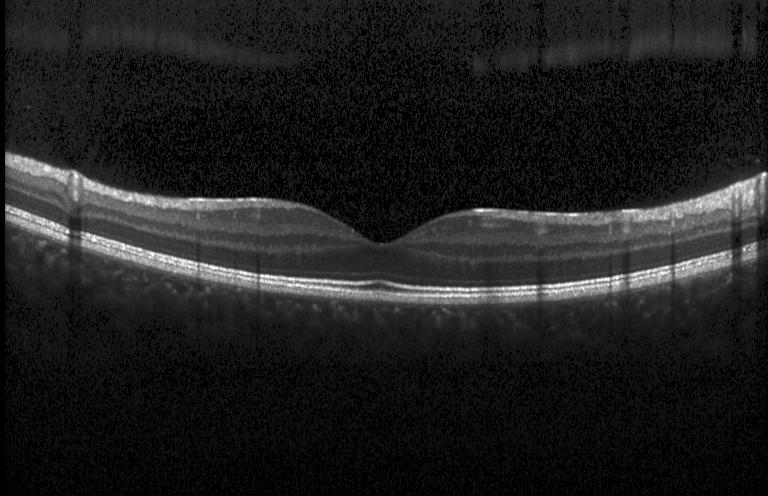
Dx: no evidence of choroidal neovascularization, diabetic macular edema, or drusen.